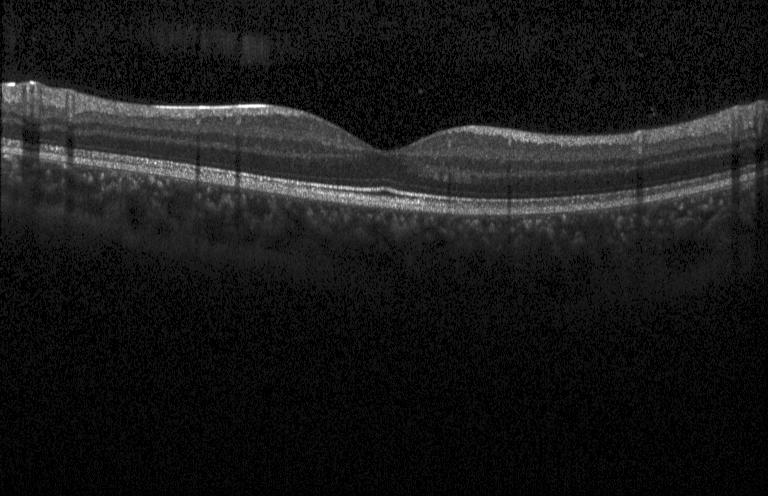

Spectral-domain optical coherence tomography. Optical coherence tomography B-scan — Impression: neither choroidal neovascularization, diabetic macular edema, nor drusen.